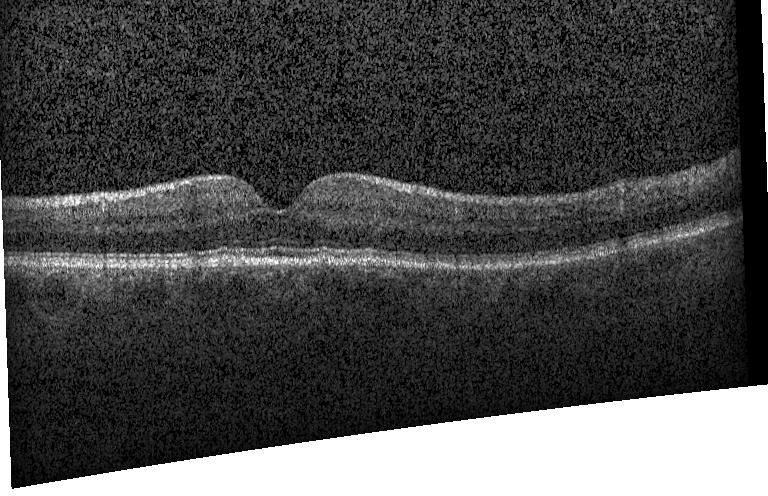

Spectral-domain optical coherence tomography · retinal OCT B-scan
Macular OCT: multiple drusen.